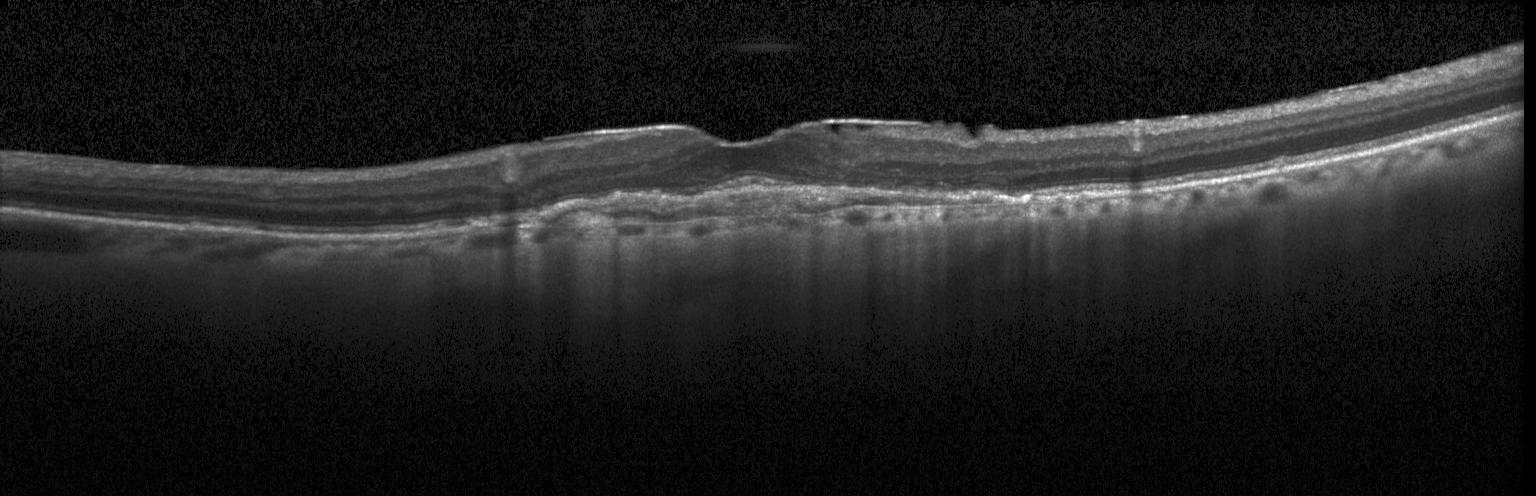 Optical coherence tomography scan, Heidelberg Spectralis, SD-OCT — Impression: a choroidal neovascular membrane.